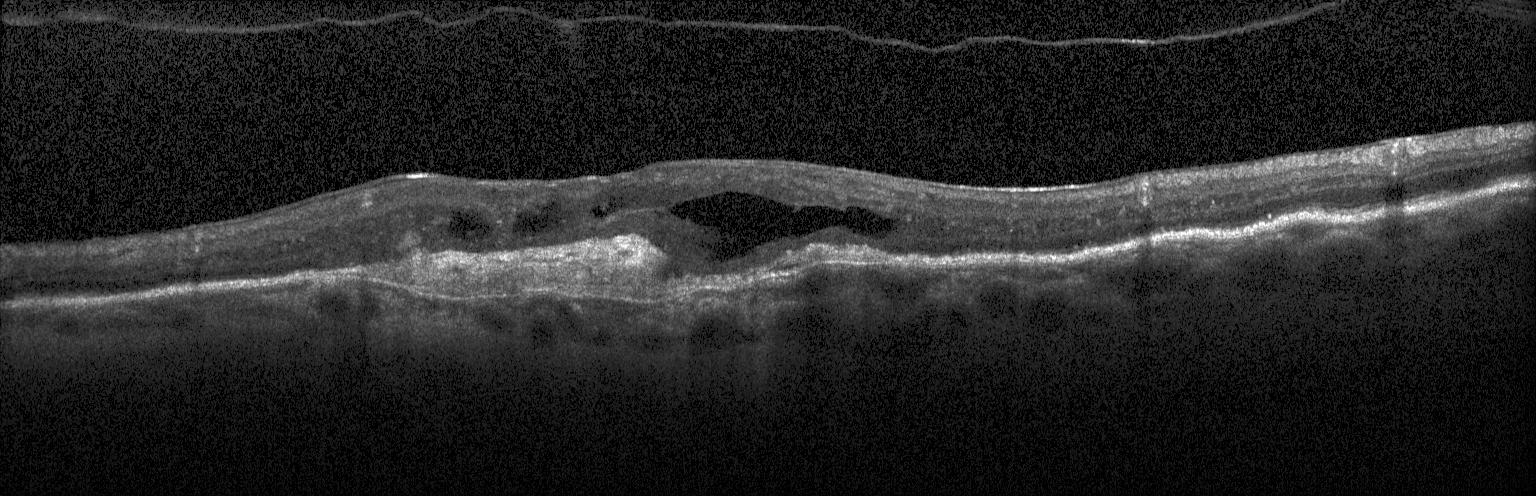 OCT finding: choroidal neovascularization (CNV).